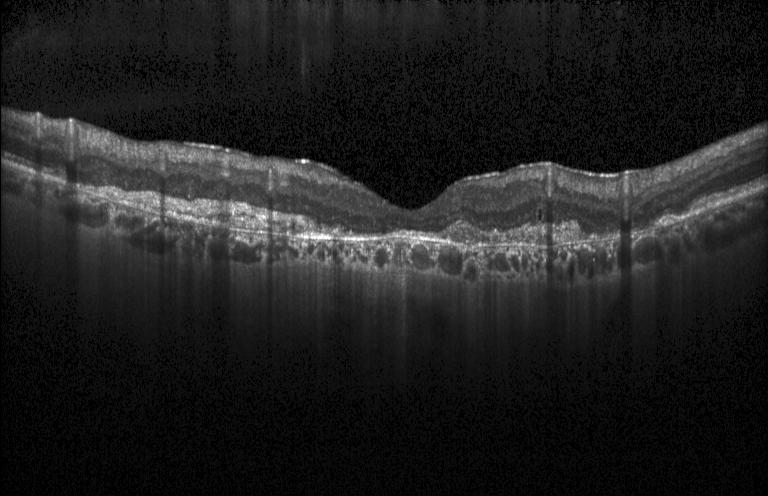

Retinal OCT B-scan · spectral-domain OCT · horizontal scan through the fovea · Heidelberg Spectralis OCT system
The scan shows a choroidal neovascular membrane.